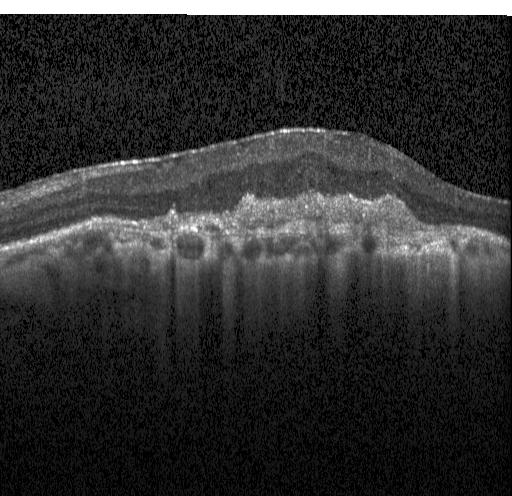 Finding: choroidal neovascularization (CNV).